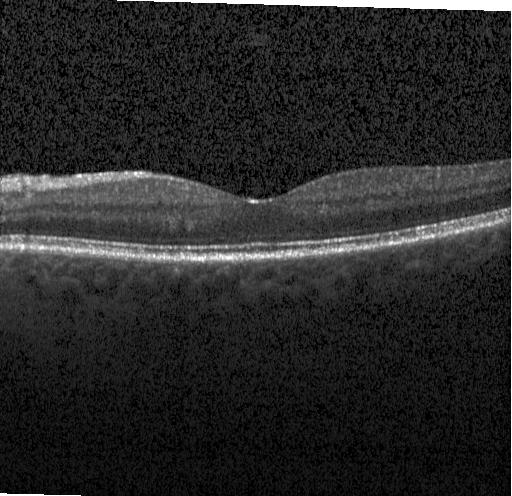

Diagnosis: no choroidal neovascularization, diabetic macular edema, or drusen.